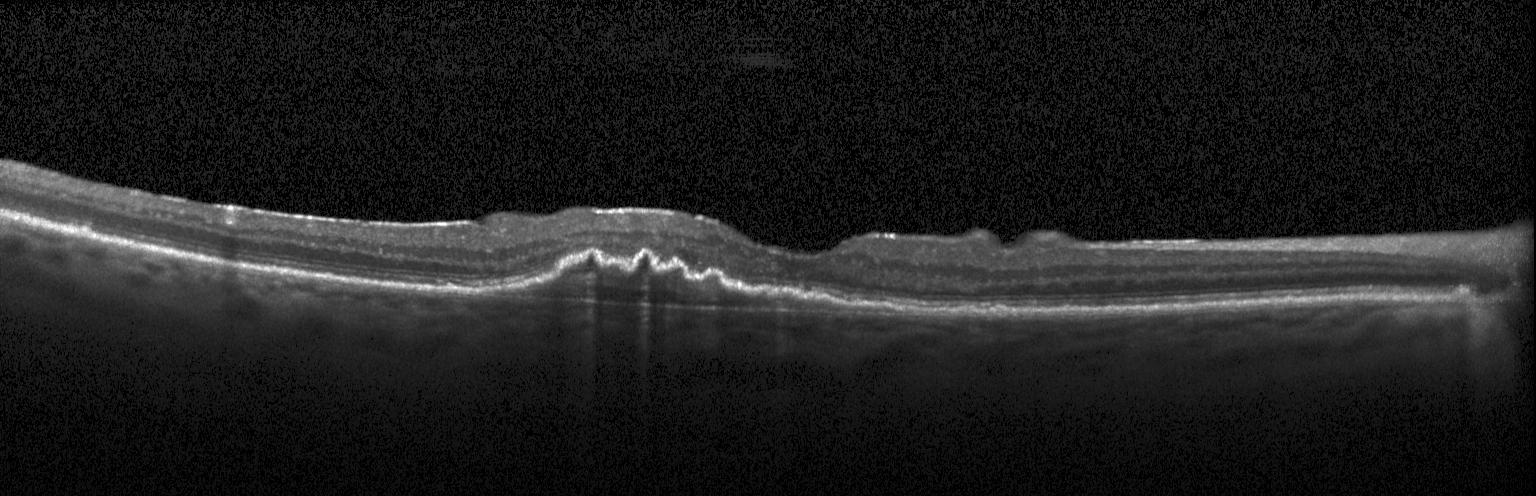

OCT B-scan · macular scan · Heidelberg Spectralis OCT system · spectral-domain optical coherence tomography.
Macular OCT: a choroidal neovascular membrane.